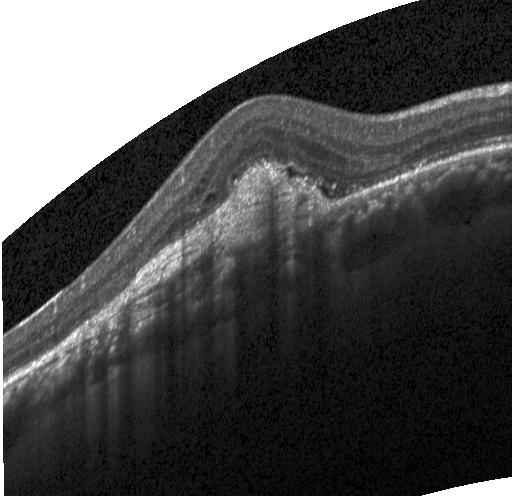 Centered on the fovea; OCT line scan; Heidelberg Spectralis OCT system; SD-OCT.
The scan shows a choroidal neovascular membrane.